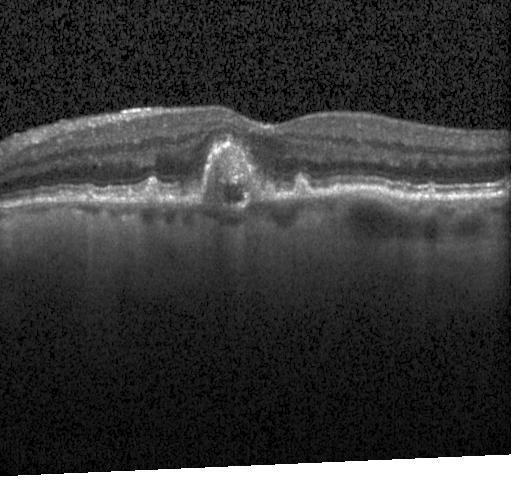 Retinal OCT cross-section · SD-OCT. Diagnosis: CNV.